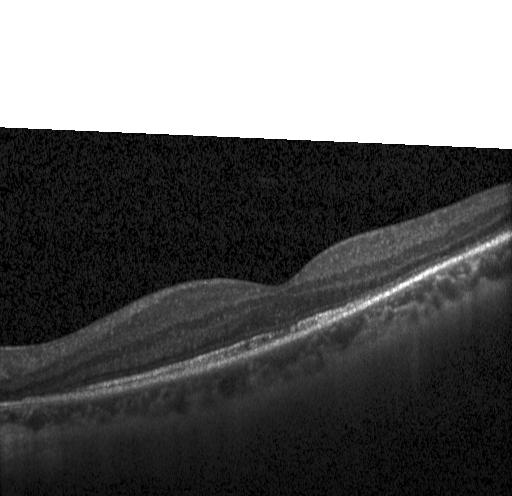 Acquired on a Heidelberg Spectralis · OCT B-scan · SD-OCT. This B-scan demonstrates no evidence of choroidal neovascularization, diabetic macular edema, or drusen.